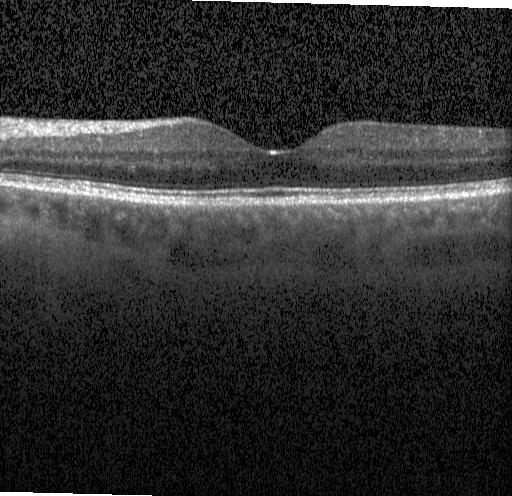 Macular OCT: neither choroidal neovascularization, diabetic macular edema, nor drusen.